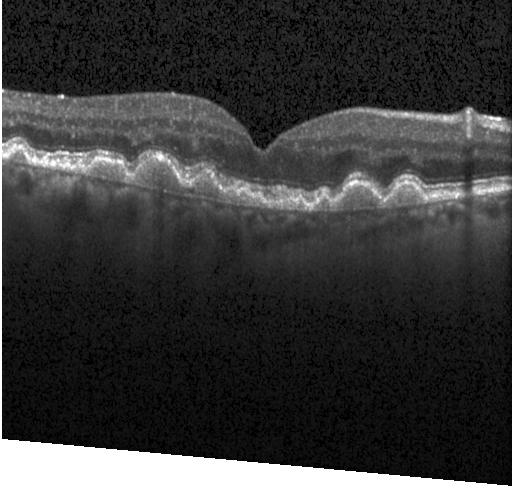

Instrument: Heidelberg Spectralis, SD-OCT, OCT line scan.
Multiple drusen.